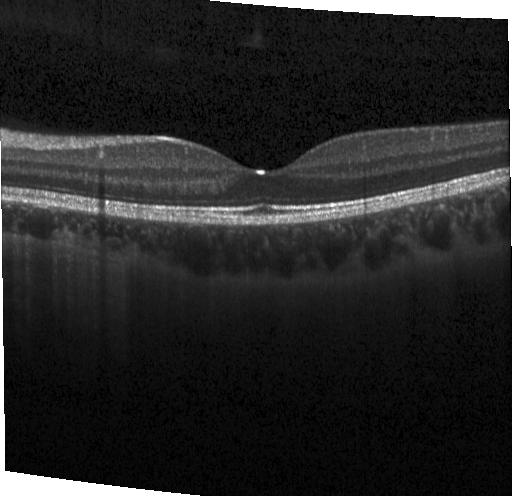
Horizontal scan through the fovea. Optical coherence tomography scan. Spectral-domain optical coherence tomography.
Assessment: no CNV, no DME, and no drusen.